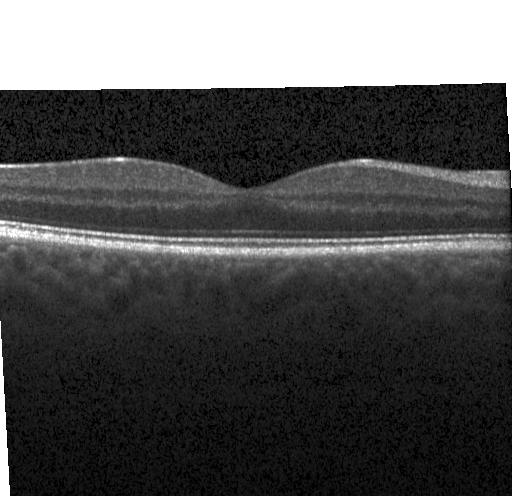

OCT scan showing no evidence of choroidal neovascularization, diabetic macular edema, or drusen.